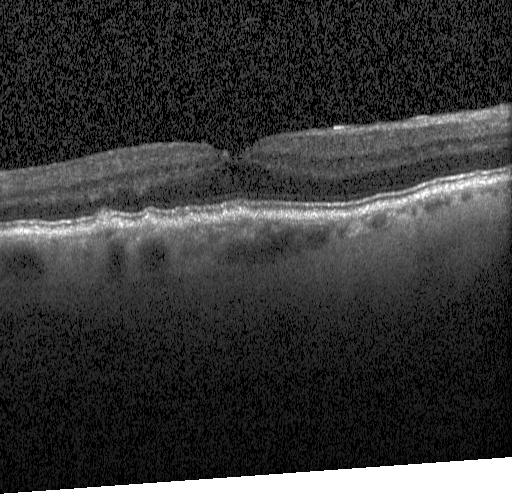

Instrument: Heidelberg Spectralis; OCT B-scan; macular scan
Macular OCT: sub-RPE drusenoid deposits.